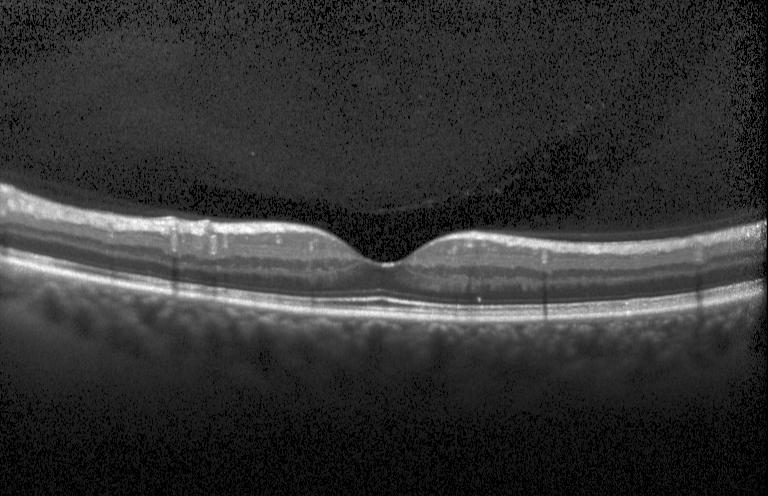 Retinal OCT cross-section.
Diagnosis: no choroidal neovascularization, no diabetic macular edema, and no drusen.